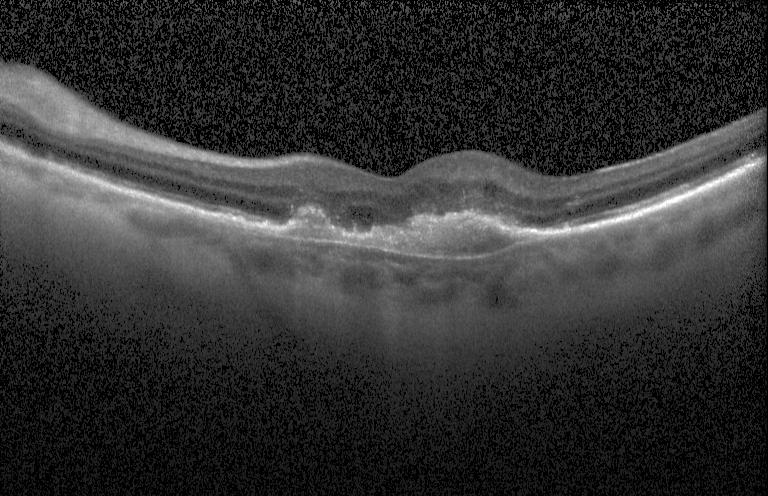
Instrument: Heidelberg Spectralis, OCT line scan, spectral-domain OCT, centered on the fovea
This B-scan demonstrates choroidal neovascularization (CNV).